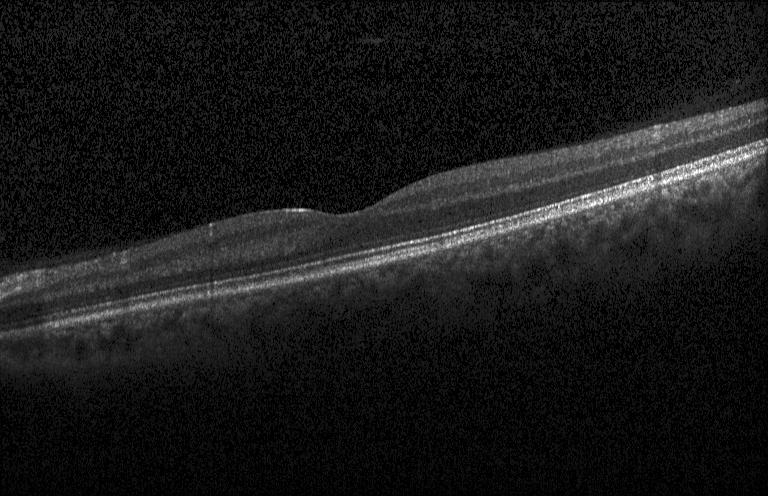
Dx: no CNV, DME, or drusen.